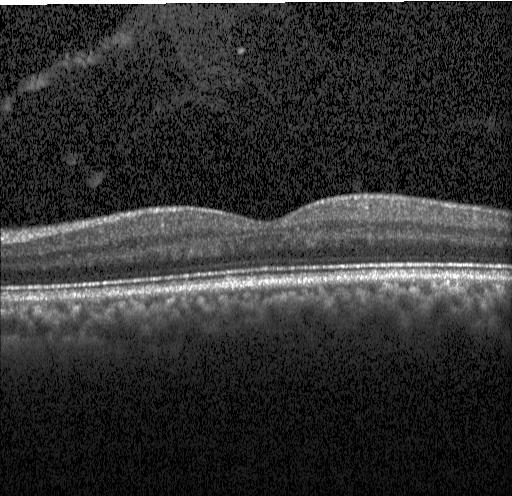 Retinal OCT B-scan. No CNV, no DME, and no drusen.